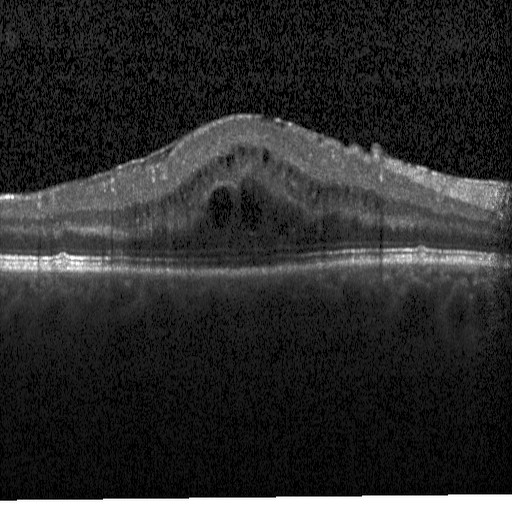
Impression: DME.